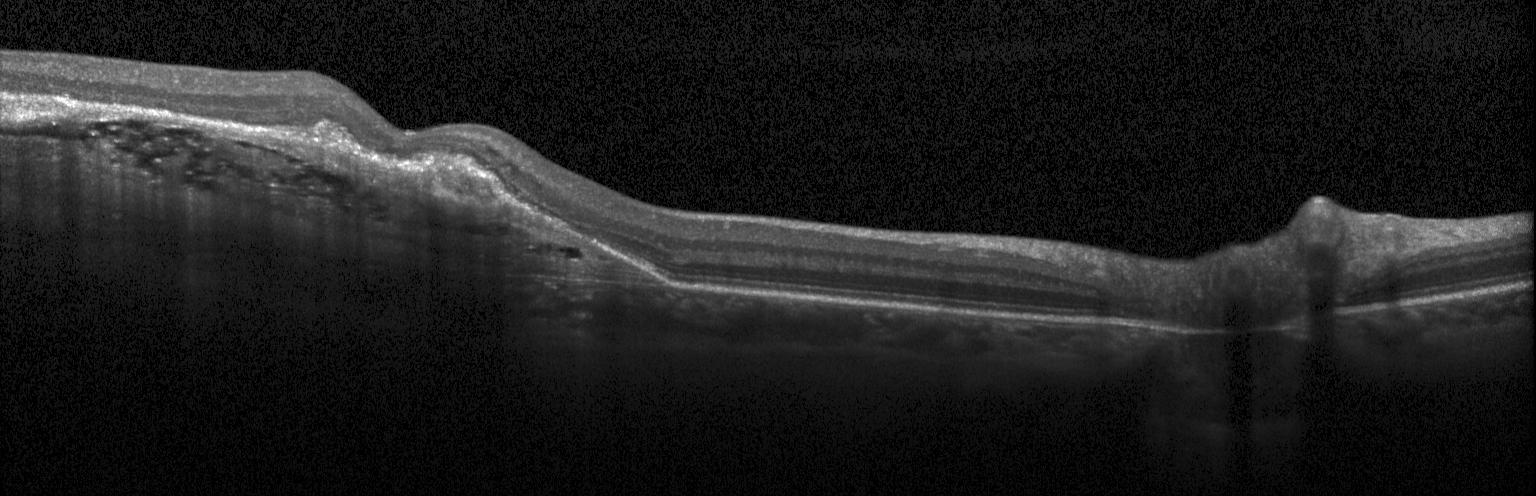
Macular OCT: a choroidal neovascular membrane.